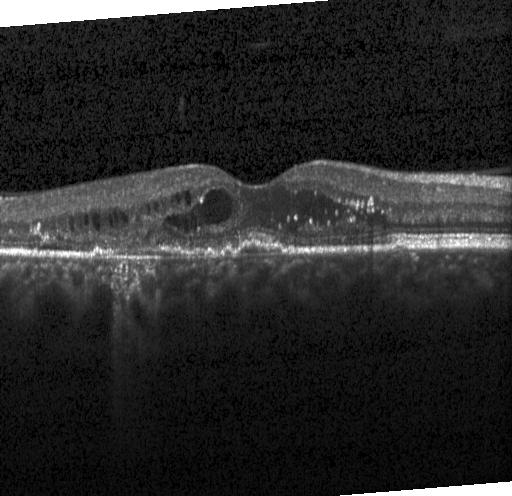
Optical coherence tomography scan · macular scan · Heidelberg Spectralis OCT system · spectral-domain optical coherence tomography — Macular OCT: choroidal neovascularization.